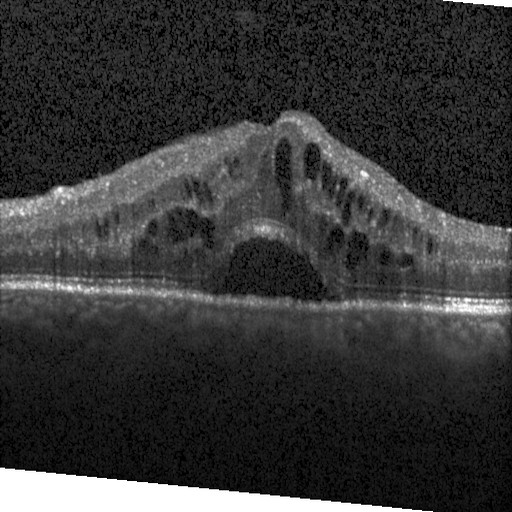

Retinal OCT B-scan. Heidelberg Spectralis. SD-OCT. Macular scan. Diabetic macular edema.